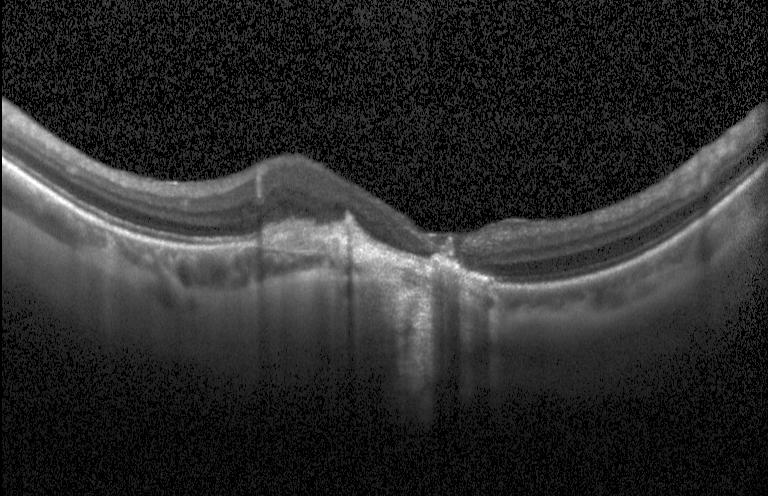 Retinal OCT cross-section.
Assessment: a choroidal neovascular membrane.